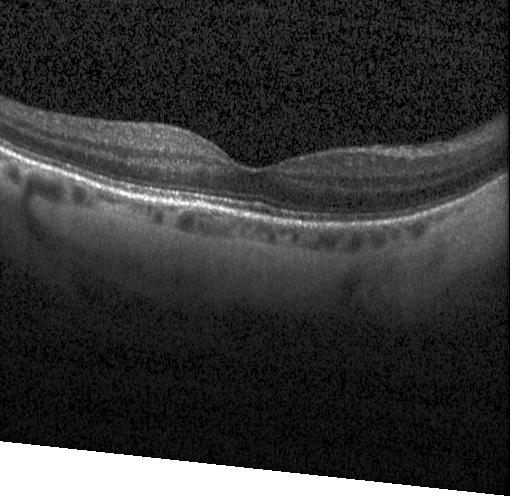

Heidelberg Spectralis, through the macula, retinal OCT B-scan — This B-scan demonstrates no evidence of CNV, DME, or drusen.